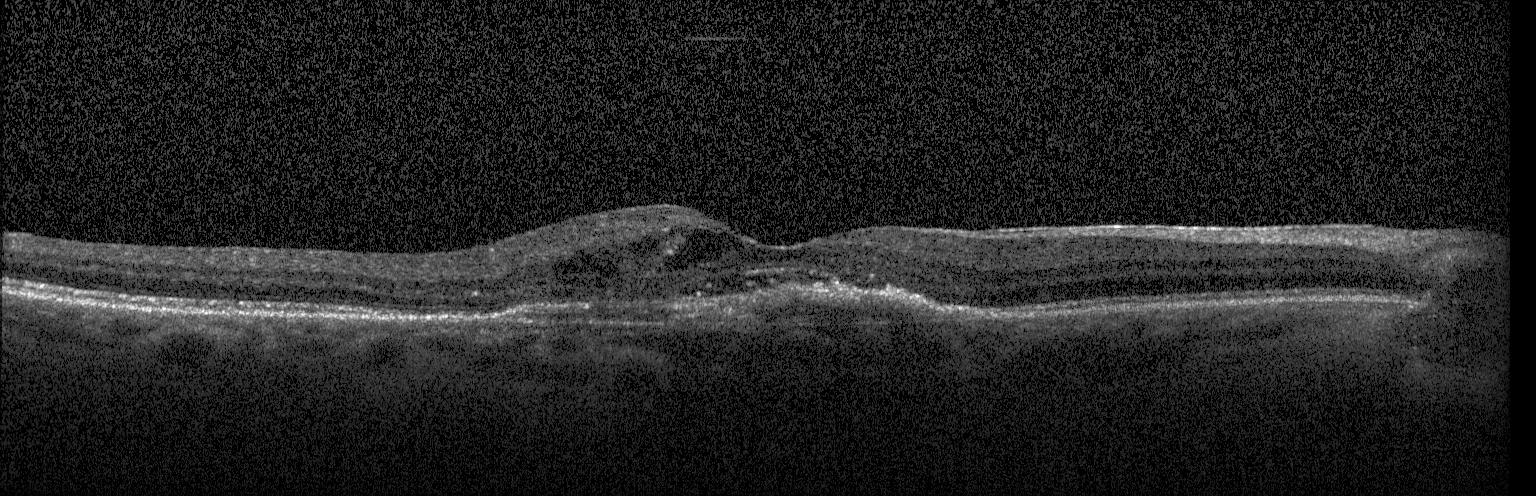 Macular OCT demonstrating CNV.